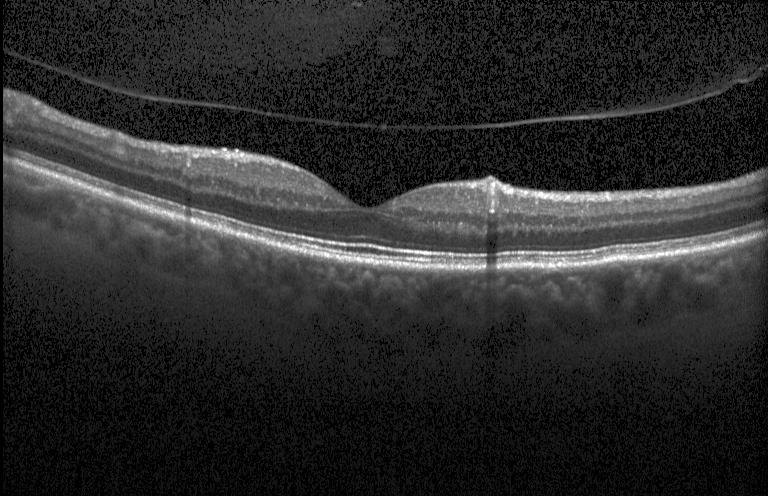 Retinal OCT B-scan. Spectral-domain optical coherence tomography. Diagnosis: neither CNV, DME, nor drusen.